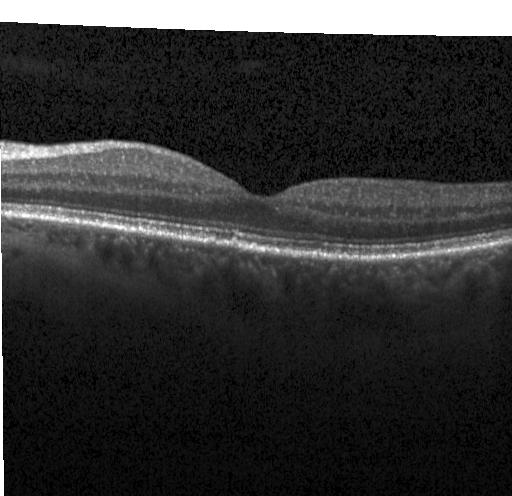

Spectral-domain OCT. Horizontal scan through the fovea. Optical coherence tomography scan. Impression: no choroidal neovascularization, diabetic macular edema, or drusen.